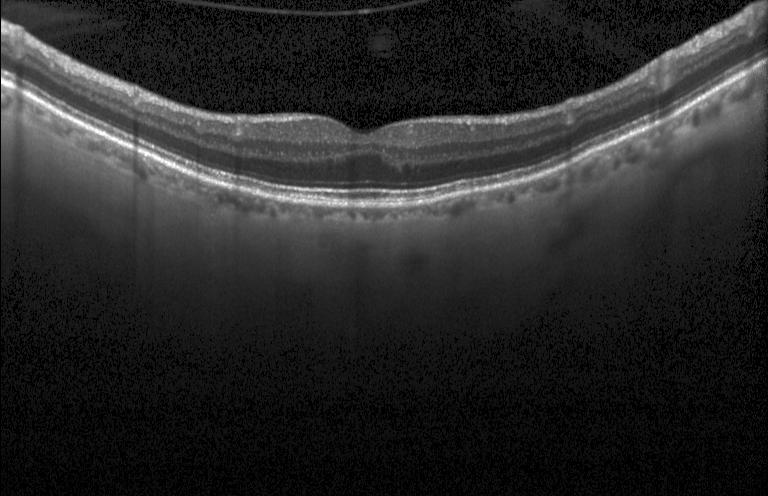

Fovea-centered. Instrument: Heidelberg Spectralis. Retinal OCT cross-section. Spectral-domain OCT
Impression: no CNV, no DME, and no drusen.